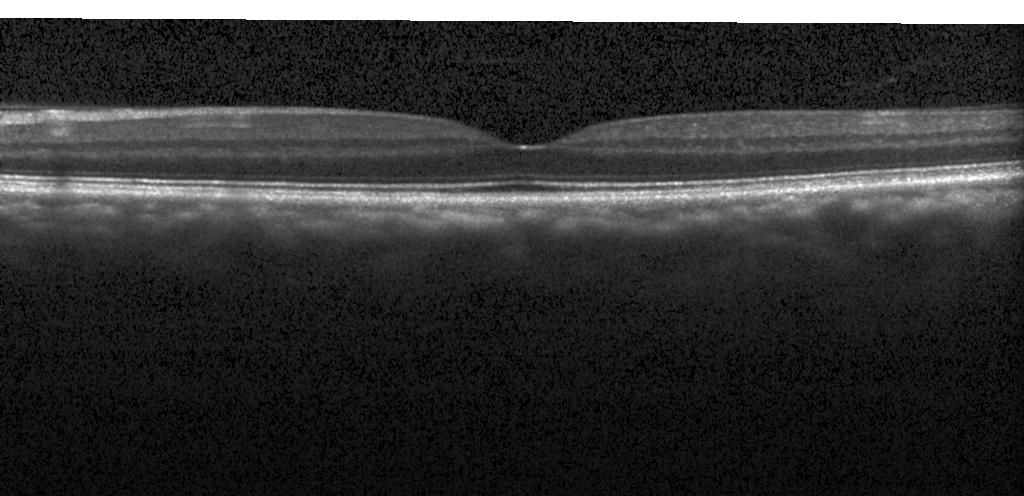

Assessment: no evidence of choroidal neovascularization, diabetic macular edema, or drusen.